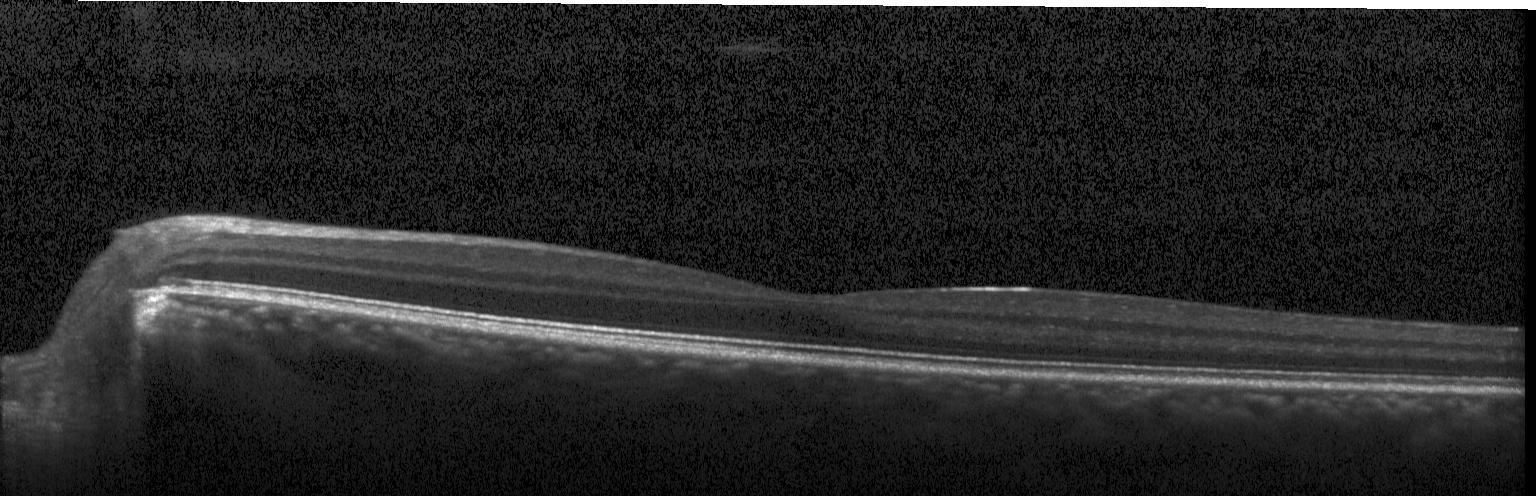

Fovea-centered; spectral-domain optical coherence tomography; retinal OCT B-scan.
The scan shows neither CNV, DME, nor drusen.